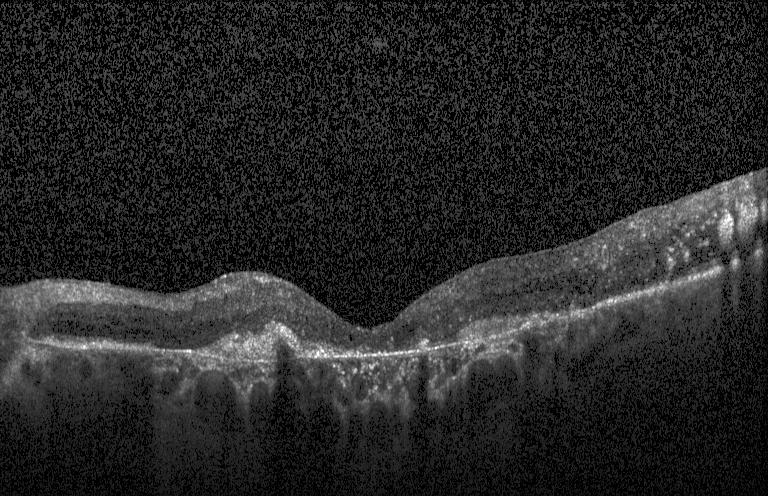 Macular scan · OCT line scan · SD-OCT · Heidelberg Spectralis.
Finding: choroidal neovascularization (CNV).